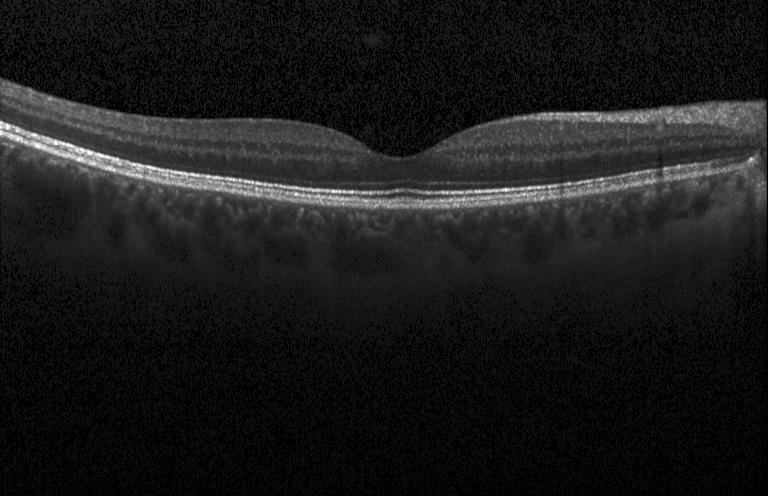
Instrument: Heidelberg Spectralis · macular scan · retinal OCT B-scan · SD-OCT — Impression: no choroidal neovascularization, diabetic macular edema, or drusen.